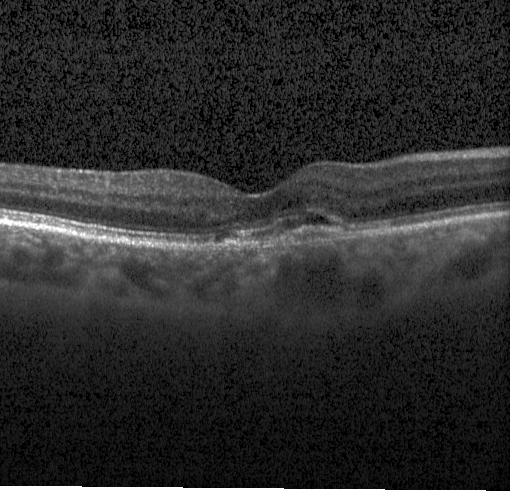 OCT line scan
Impression: a choroidal neovascular membrane.